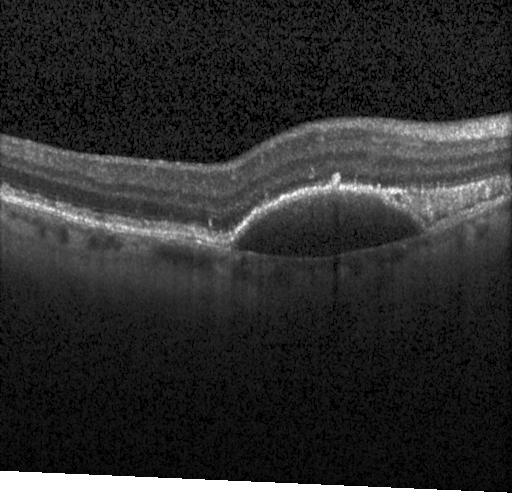

Retinal OCT B-scan; acquired on a Heidelberg Spectralis.
Dx: choroidal neovascularization (CNV).